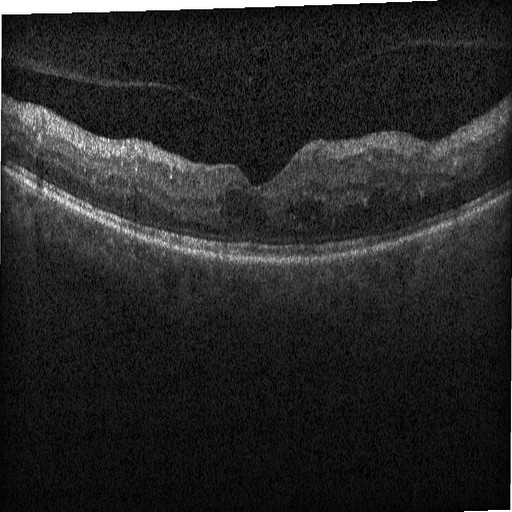 OCT finding: diabetic macular edema (DME).